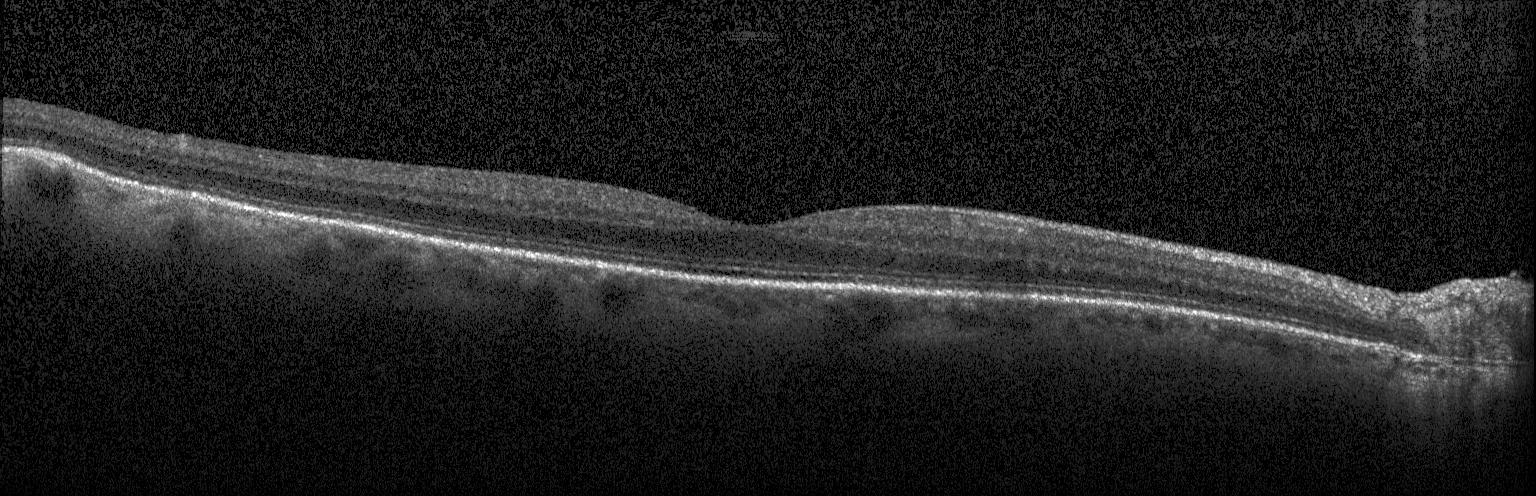 Retinal OCT B-scan, through the macula.
Finding: neither choroidal neovascularization, diabetic macular edema, nor drusen.